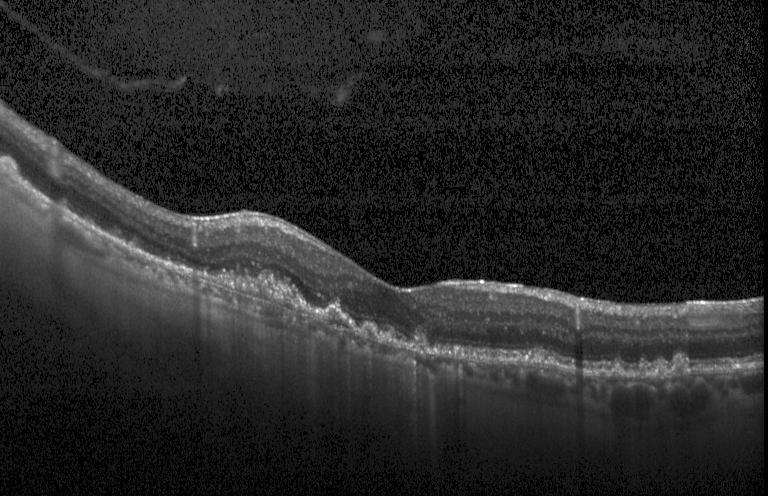

Macular OCT: CNV.